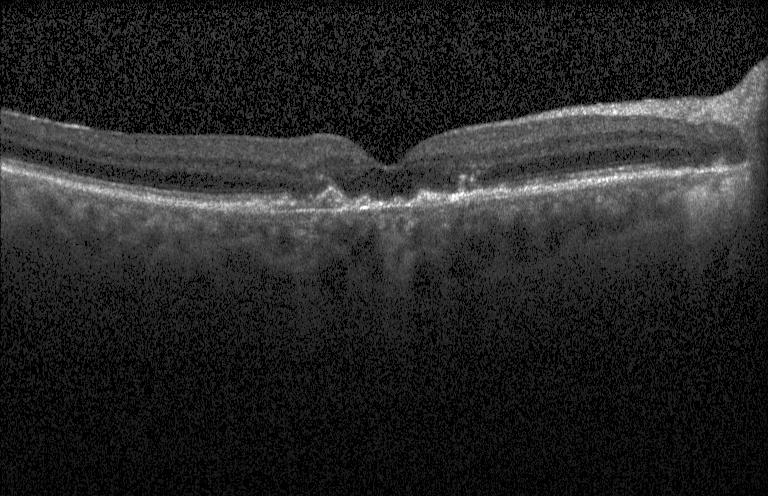
This B-scan demonstrates a choroidal neovascular membrane.